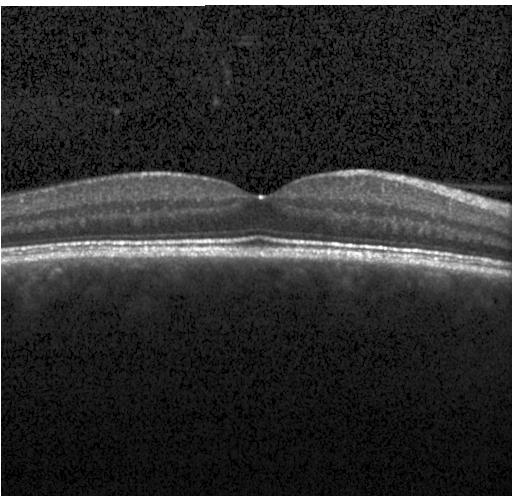 Horizontal scan through the fovea, optical coherence tomography scan, SD-OCT — The scan shows no evidence of choroidal neovascularization, diabetic macular edema, or drusen.